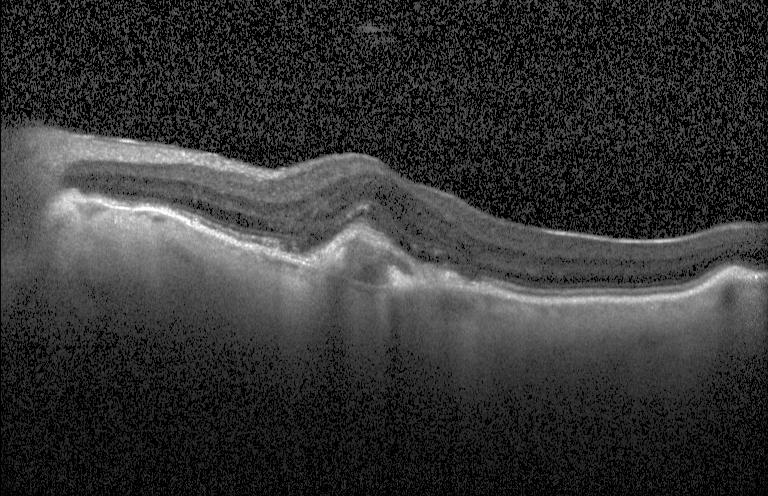 Macular OCT: choroidal neovascularization (CNV).